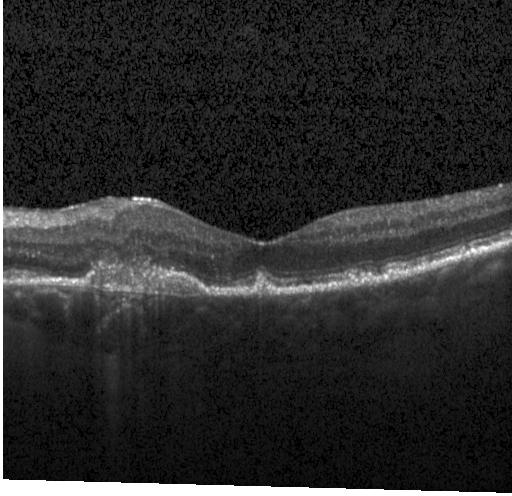

Heidelberg Spectralis OCT system · optical coherence tomography scan — The scan shows choroidal neovascularization.